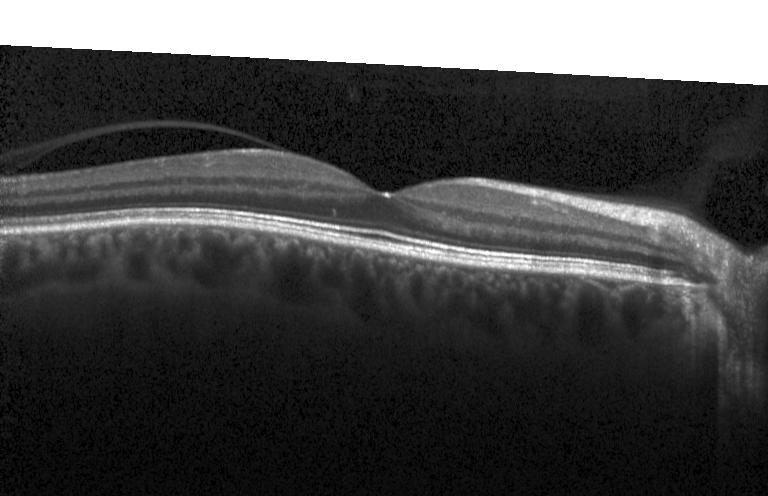
Finding: no evidence of choroidal neovascularization, diabetic macular edema, or drusen.